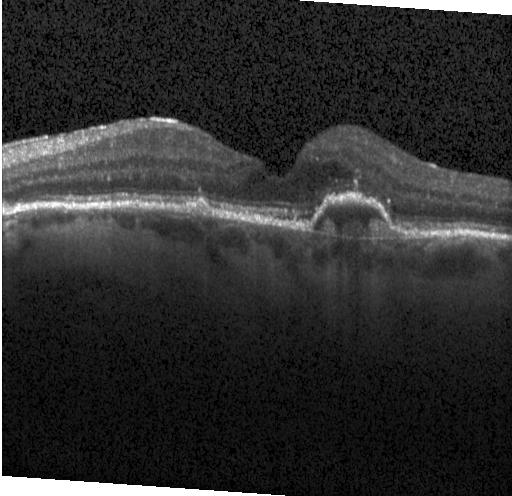

Diagnosis: a choroidal neovascular membrane.